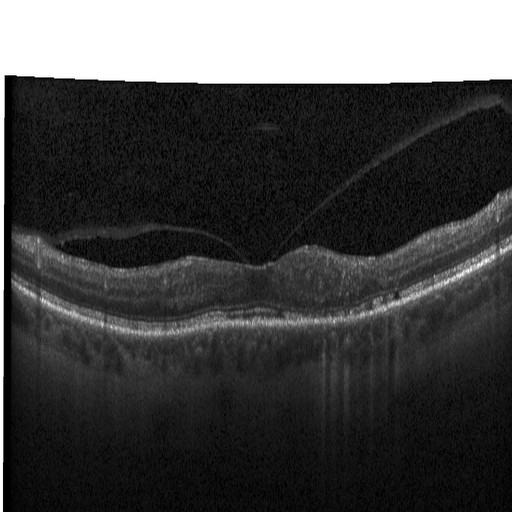
Diagnosis: diabetic macular edema.